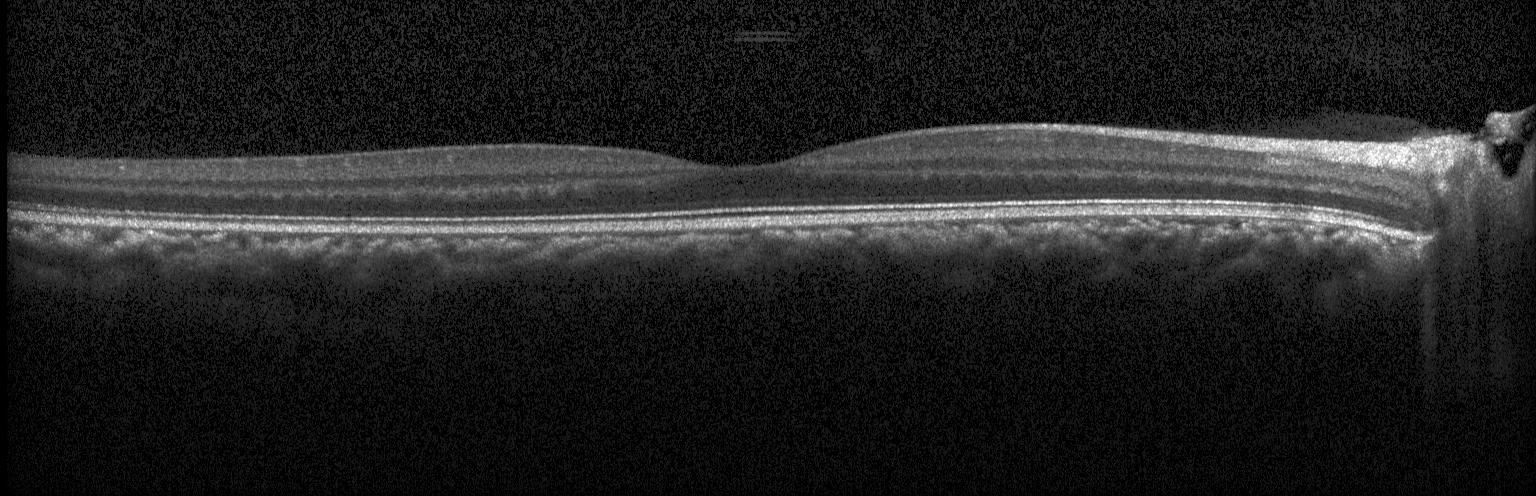

Fovea-centered · optical coherence tomography B-scan.
Finding: no choroidal neovascularization, diabetic macular edema, or drusen.